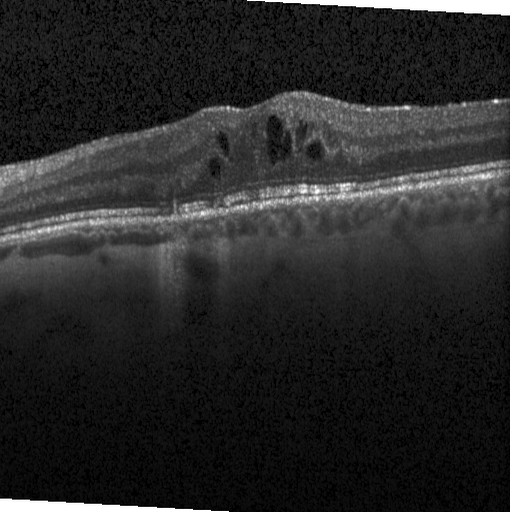
Horizontal scan through the fovea, OCT B-scan
Diabetic macular edema (DME).